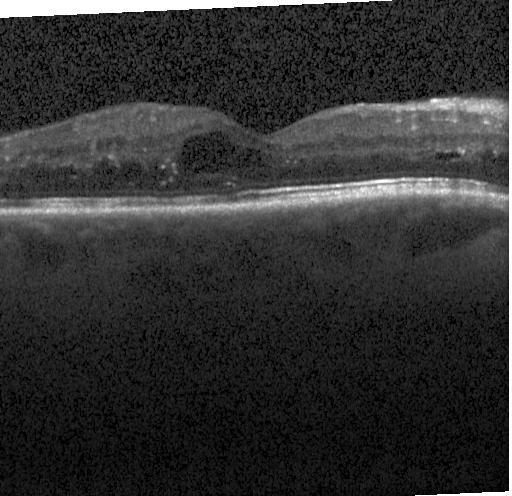 Acquired on a Heidelberg Spectralis · retinal OCT cross-section.
The scan shows diabetic macular edema (DME).